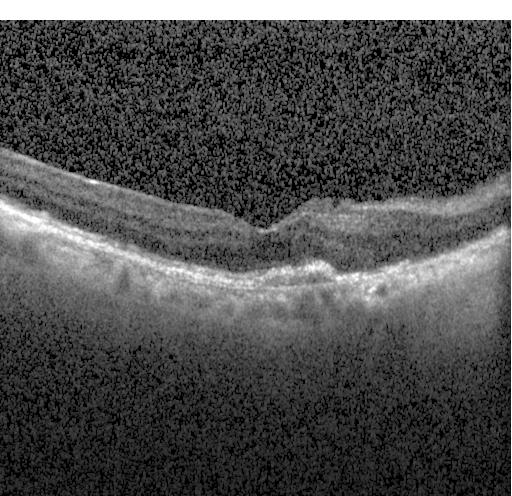 Heidelberg Spectralis OCT system; OCT line scan — Finding: CNV.